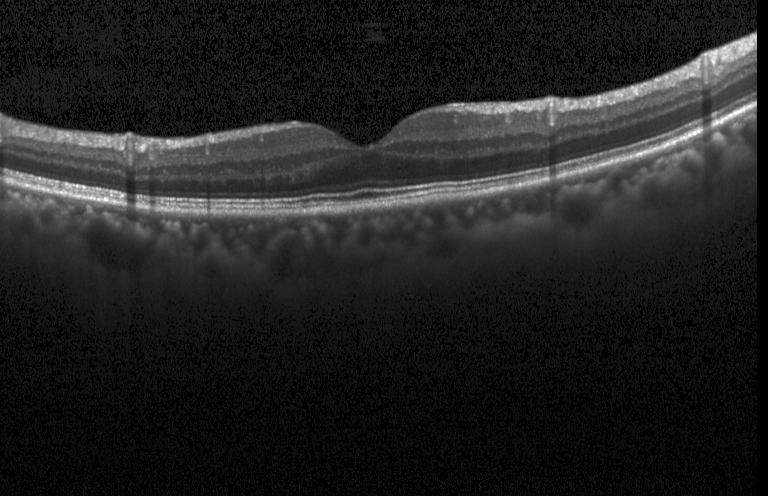 Optical coherence tomography B-scan — OCT finding: no evidence of choroidal neovascularization, diabetic macular edema, or drusen.